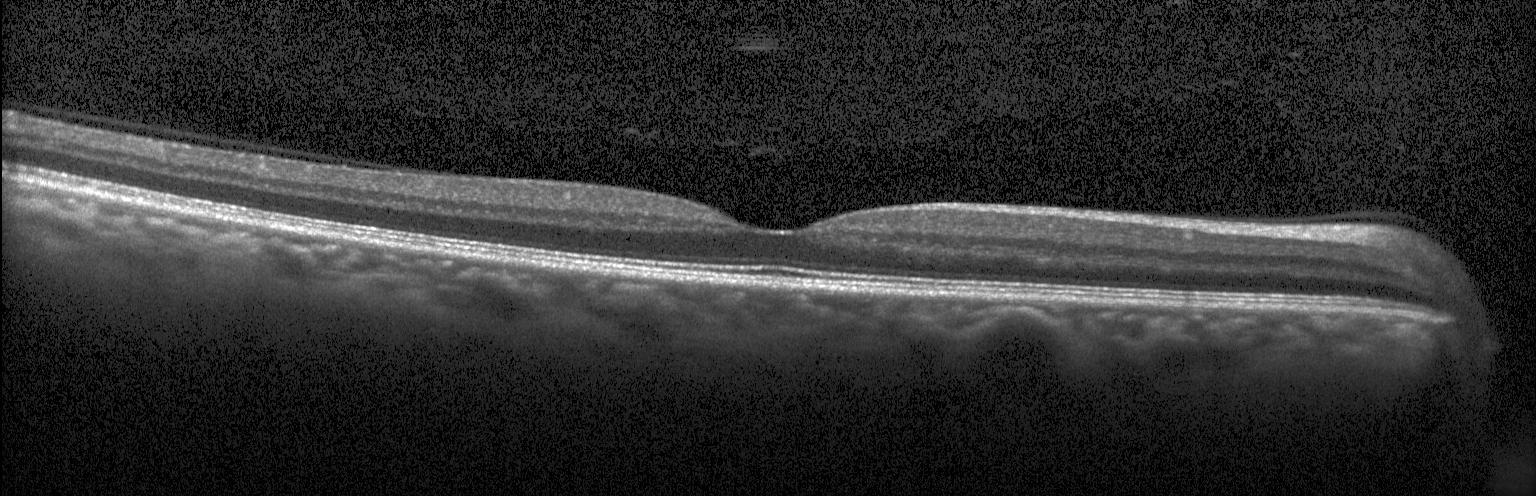 OCT B-scan. Dx: neither choroidal neovascularization, diabetic macular edema, nor drusen.